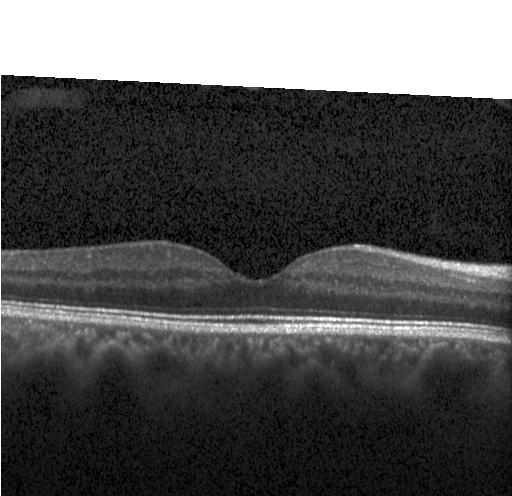 SD-OCT, OCT line scan — Dx: no choroidal neovascularization, no diabetic macular edema, and no drusen.